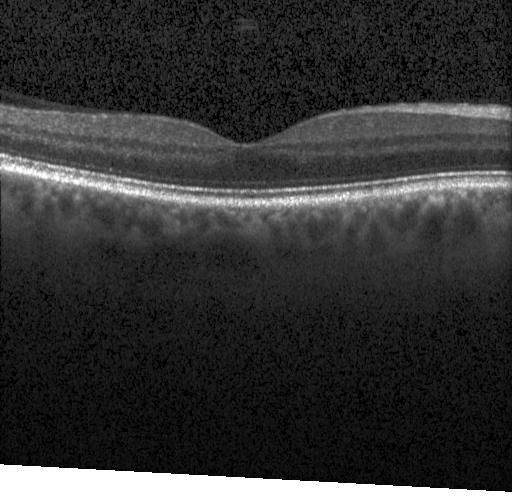
Retinal OCT B-scan; macular scan; instrument: Heidelberg Spectralis; spectral-domain OCT — Macular OCT: no CNV, no DME, and no drusen.